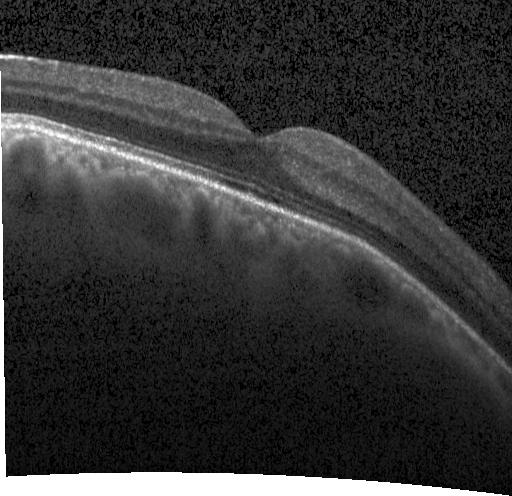
Heidelberg Spectralis · optical coherence tomography scan · SD-OCT — The scan shows neither choroidal neovascularization, diabetic macular edema, nor drusen.